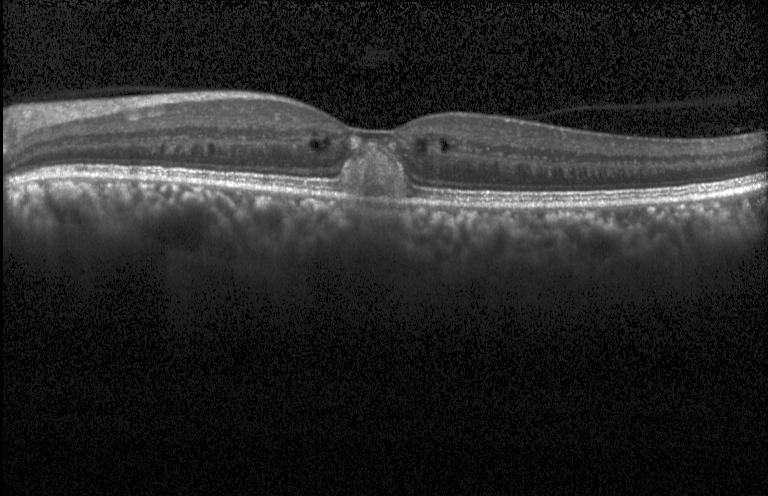
Retinal OCT B-scan. Spectral-domain optical coherence tomography. Macular scan
Choroidal neovascularization (CNV).